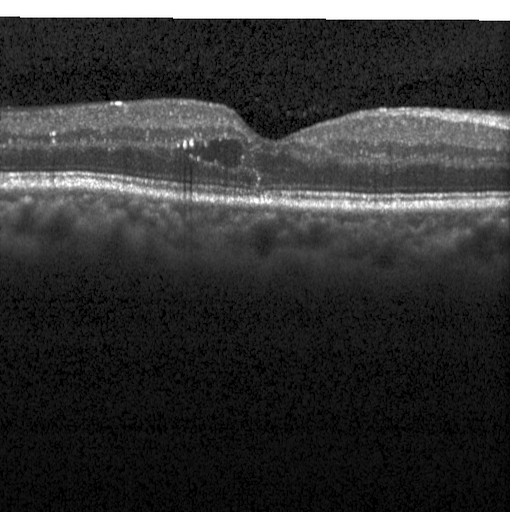 Dx: diabetic macular edema.